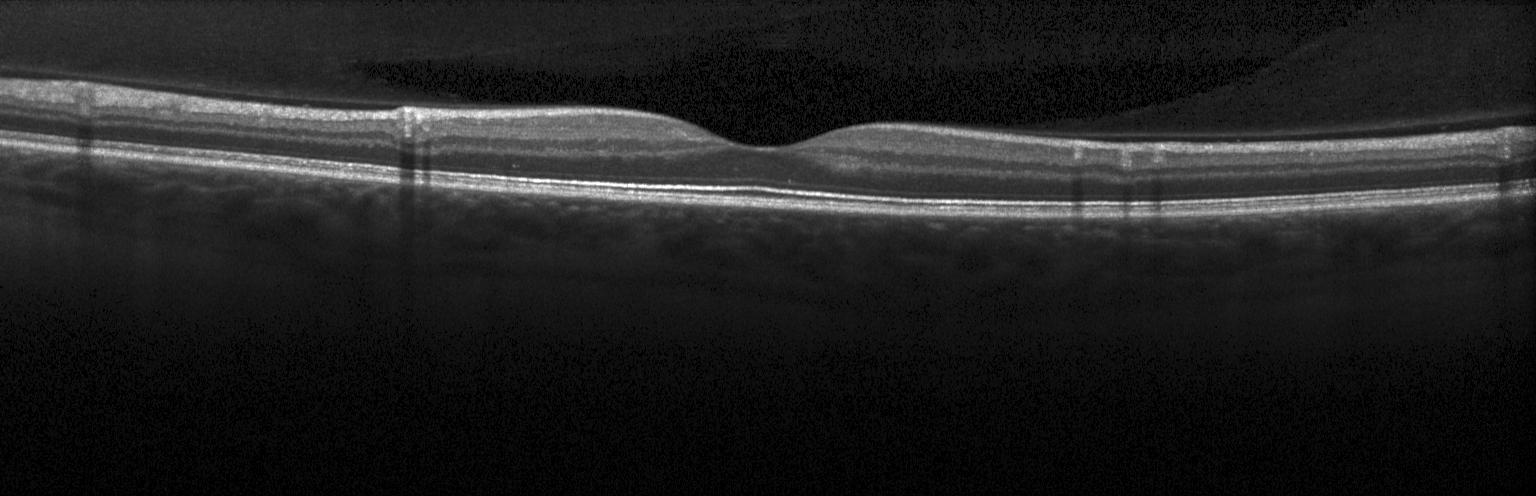 OCT line scan — No choroidal neovascularization, diabetic macular edema, or drusen.